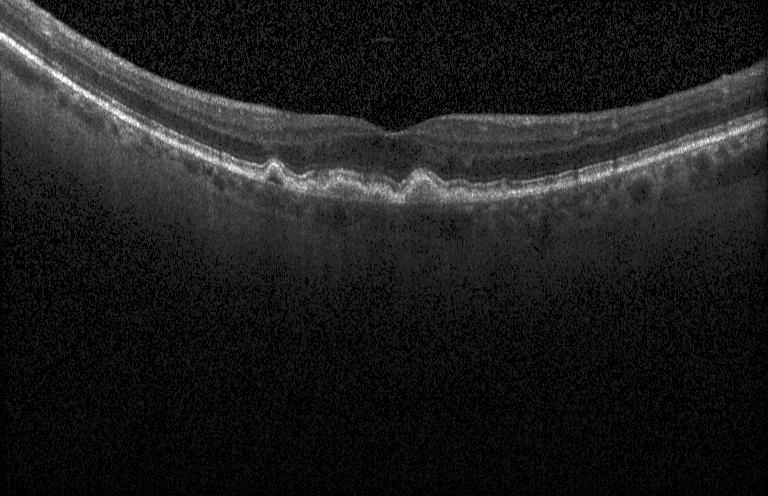

SD-OCT, retinal OCT cross-section, instrument: Heidelberg Spectralis, centered on the fovea. Multiple drusen.